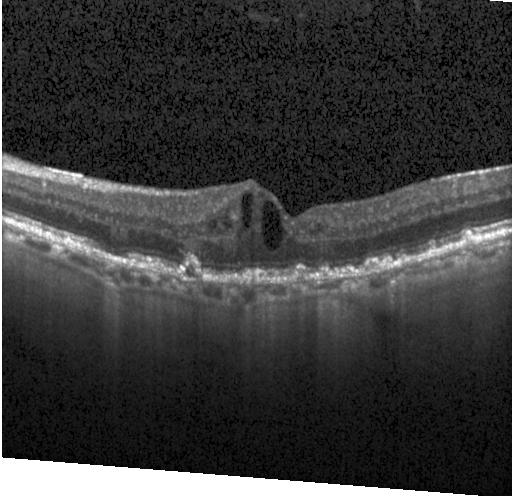 Dx: a choroidal neovascular membrane.